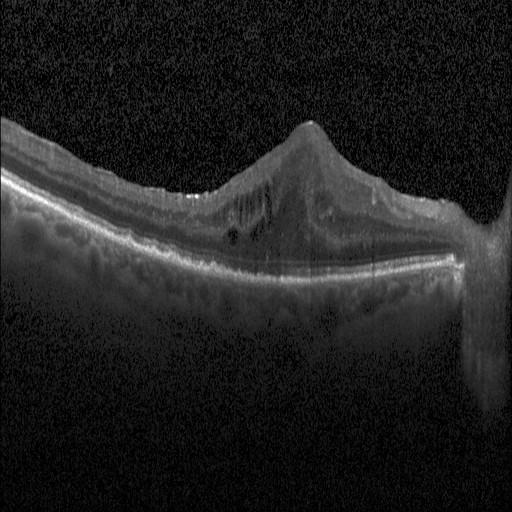 Spectral-domain OCT B-scan: DME.